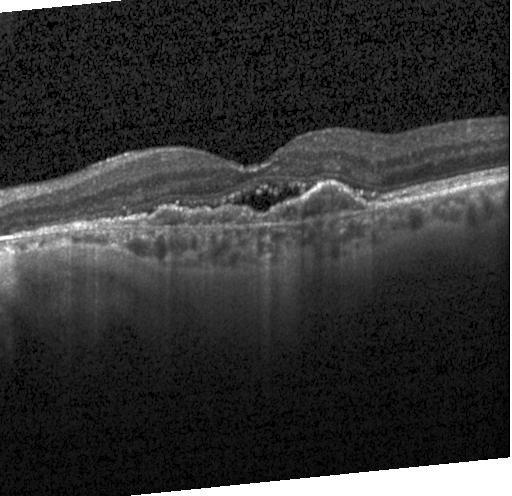

Retinal OCT B-scan — The scan shows a choroidal neovascular membrane.